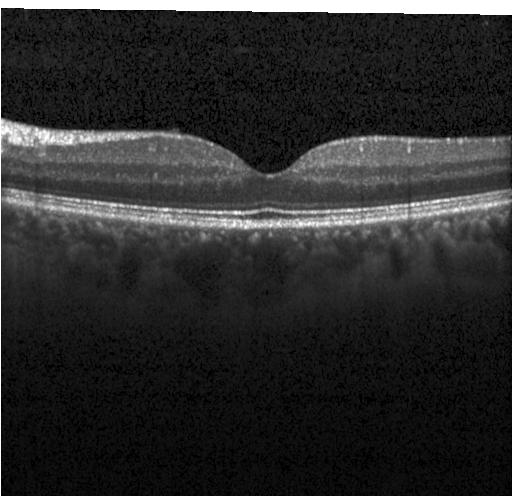
Diagnosis: no evidence of CNV, DME, or drusen.